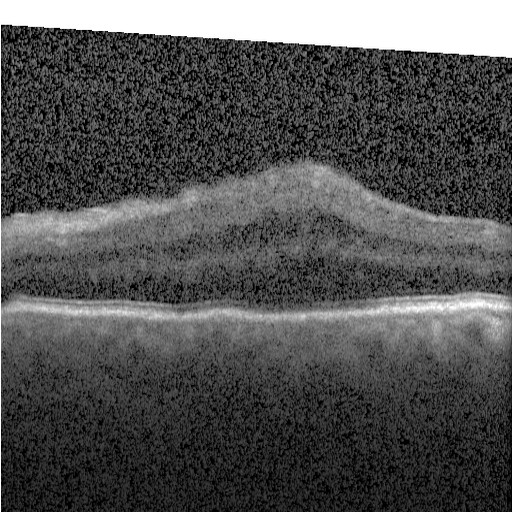

Spectral-domain optical coherence tomography; retinal OCT cross-section
Assessment: DME.